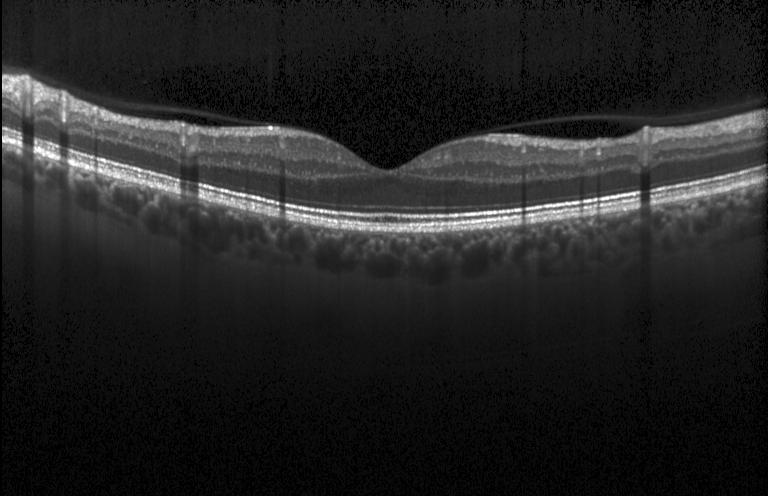
Retinal OCT B-scan. Acquired on a Heidelberg Spectralis — No CNV, DME, or drusen.